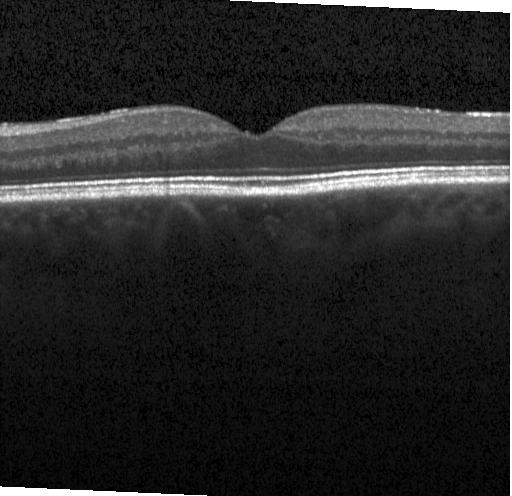 Macular OCT demonstrating no choroidal neovascularization, diabetic macular edema, or drusen.